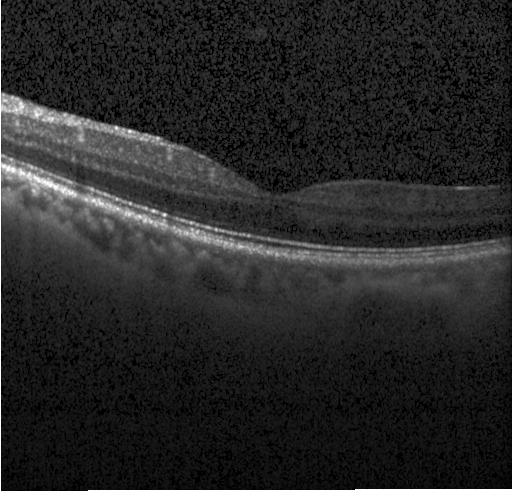 Finding: no evidence of choroidal neovascularization, diabetic macular edema, or drusen.